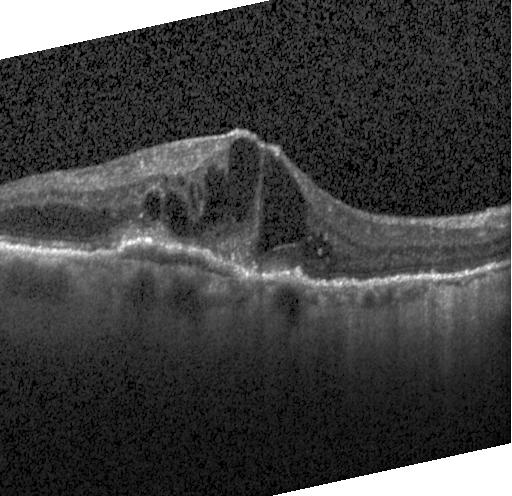 Optical coherence tomography scan; instrument: Heidelberg Spectralis.
This B-scan demonstrates a choroidal neovascular membrane.